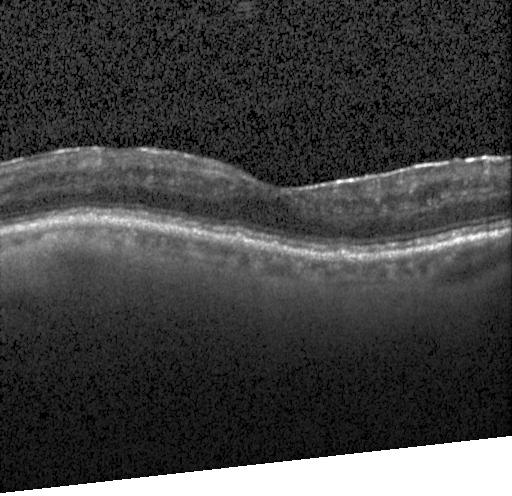 Spectral-domain OCT, retinal OCT cross-section, through the macula. Finding: multiple drusen.